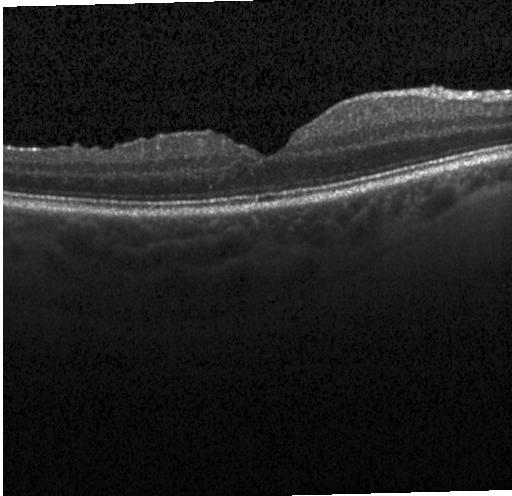

Impression: no choroidal neovascularization, no diabetic macular edema, and no drusen.